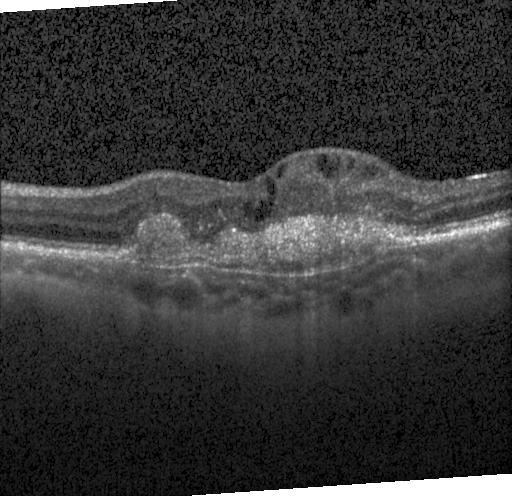

Optical coherence tomography B-scan. Assessment: a choroidal neovascular membrane.